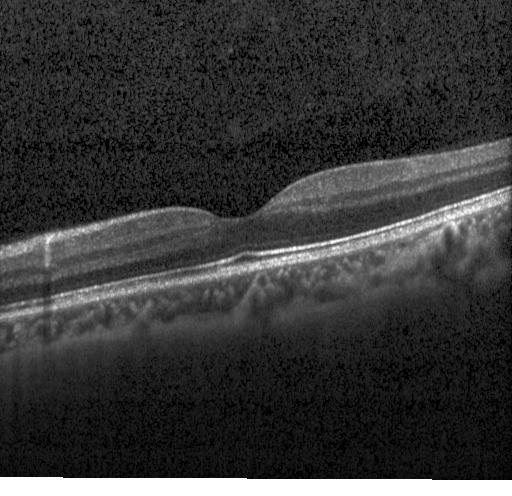
Spectral-domain optical coherence tomography, macular scan, optical coherence tomography scan, Heidelberg Spectralis — Diagnosis: no evidence of choroidal neovascularization, diabetic macular edema, or drusen.